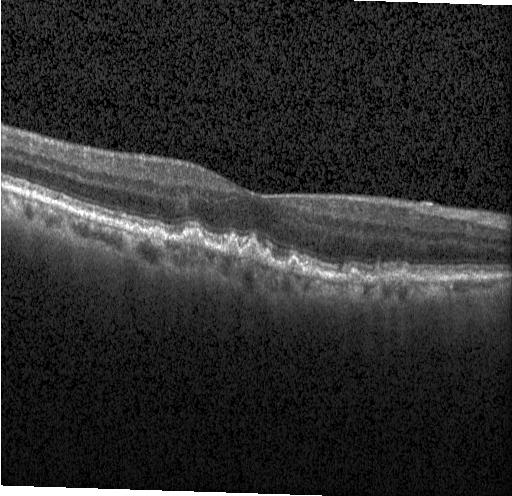
Instrument: Heidelberg Spectralis · optical coherence tomography B-scan. Finding: sub-RPE drusenoid deposits.